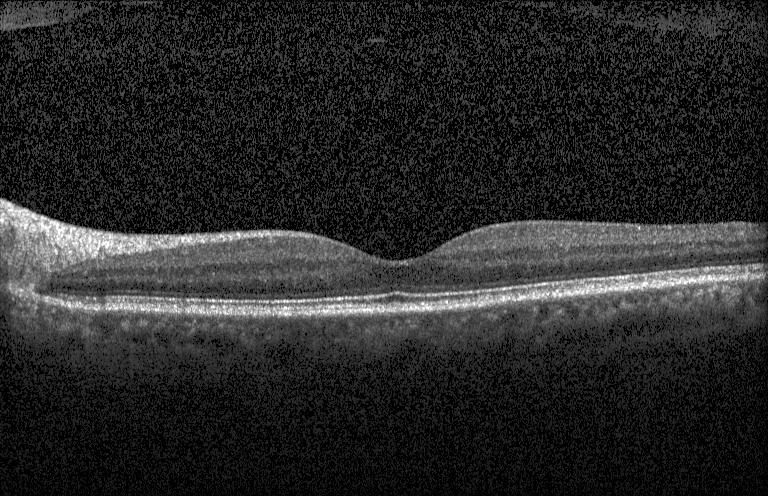

Macular OCT demonstrating neither choroidal neovascularization, diabetic macular edema, nor drusen.